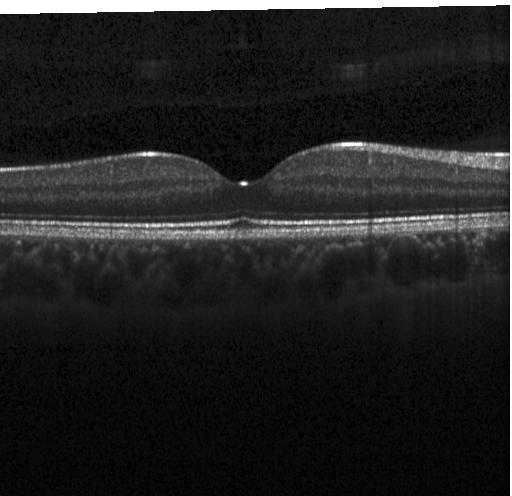
Retinal OCT B-scan.
Dx: no evidence of choroidal neovascularization, diabetic macular edema, or drusen.